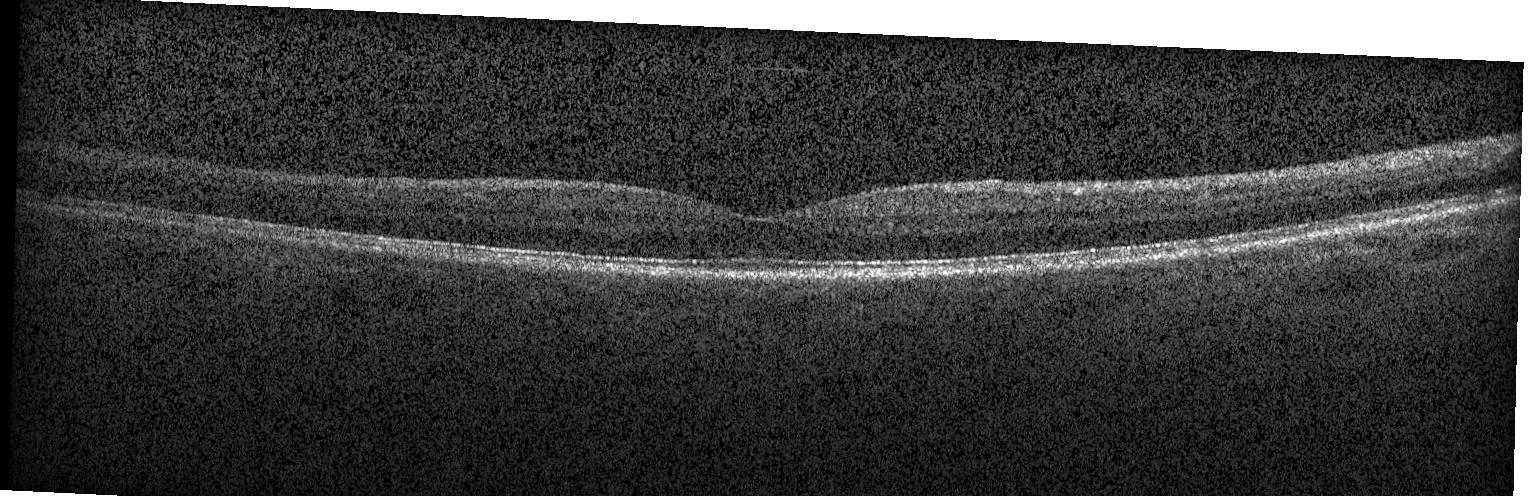 OCT line scan. Spectral-domain OCT. Centered on the fovea. Instrument: Heidelberg Spectralis. This B-scan demonstrates no choroidal neovascularization, diabetic macular edema, or drusen.